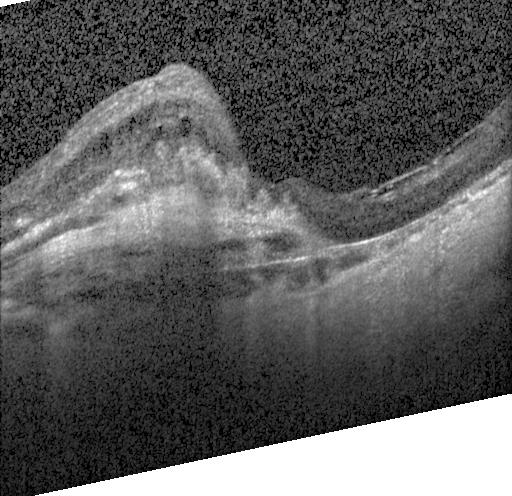 OCT line scan — Diagnosis: choroidal neovascularization (CNV).